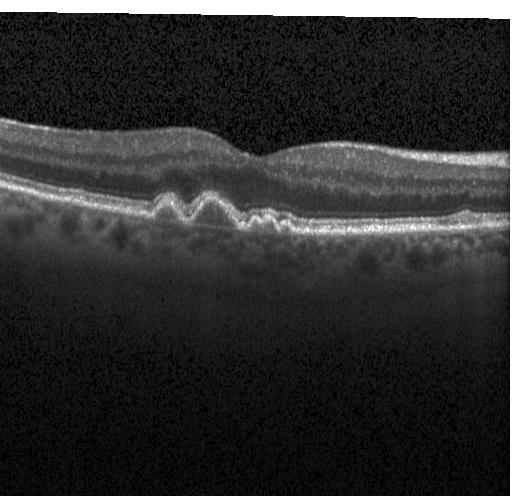

Horizontal scan through the fovea. Retinal OCT B-scan. Assessment: multiple drusen.